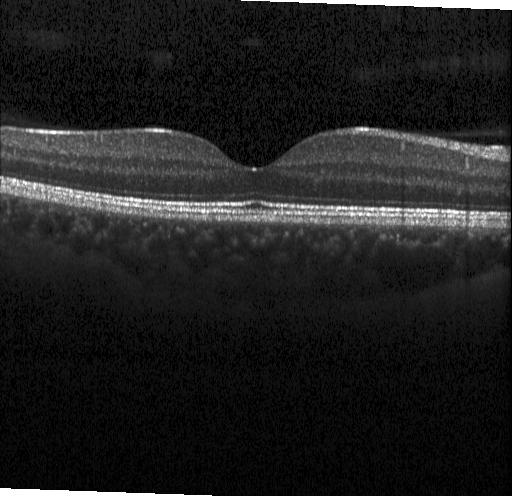

Optical coherence tomography B-scan · fovea-centered — The scan shows no CNV, DME, or drusen.